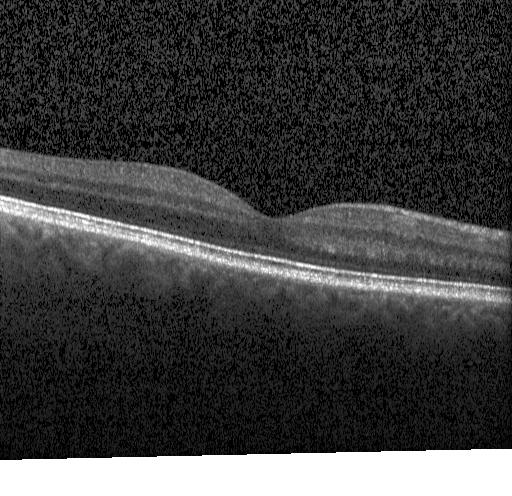 Spectral-domain OCT; optical coherence tomography B-scan
Diagnosis: neither choroidal neovascularization, diabetic macular edema, nor drusen.